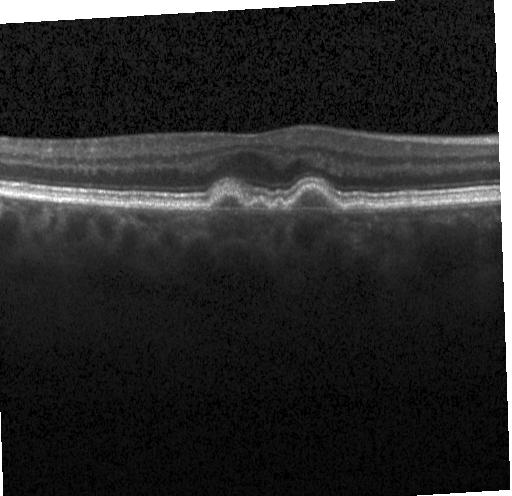
Fovea-centered, acquired on a Heidelberg Spectralis, spectral-domain OCT, optical coherence tomography B-scan. OCT finding: sub-RPE drusenoid deposits.